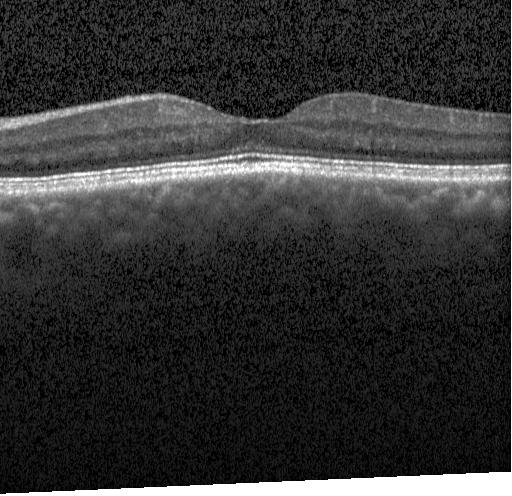
SD-OCT · retinal OCT cross-section. Impression: no choroidal neovascularization, diabetic macular edema, or drusen.